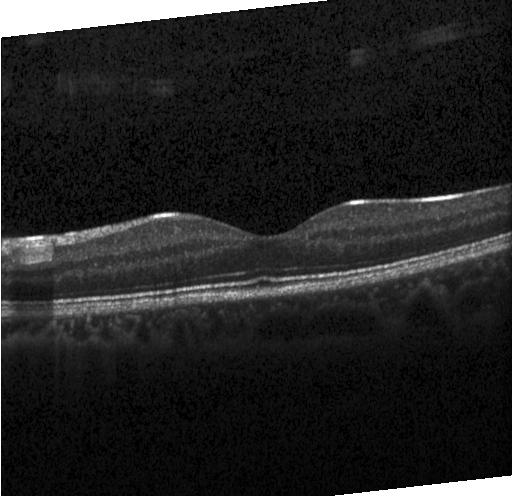
Macular OCT demonstrating no choroidal neovascularization, diabetic macular edema, or drusen.